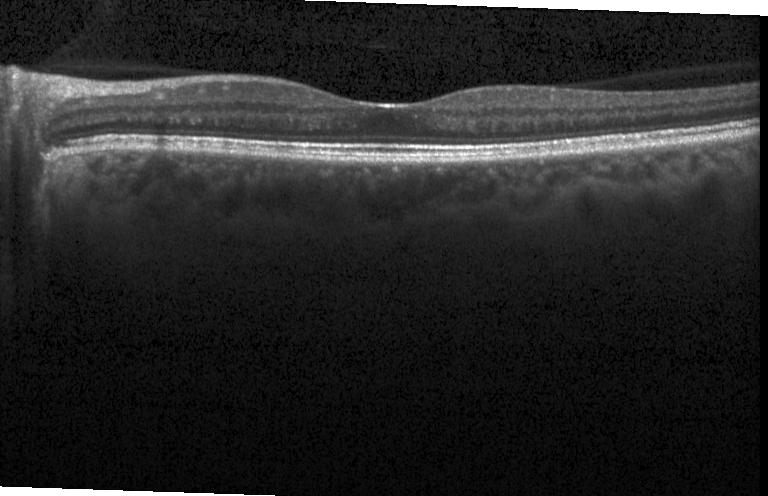
SD-OCT. OCT line scan.
Finding: no CNV, DME, or drusen.